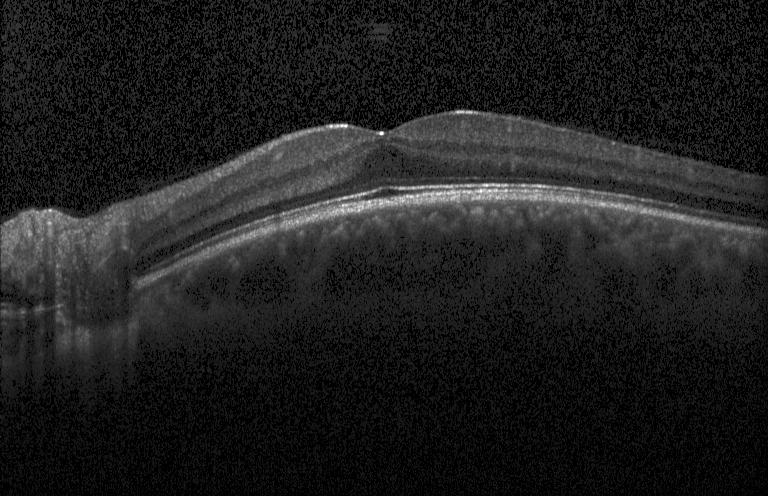 Impression: neither choroidal neovascularization, diabetic macular edema, nor drusen.